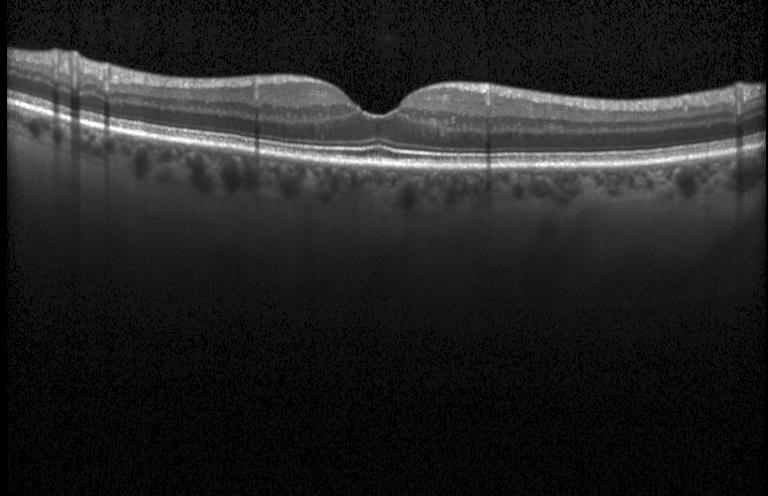

Retinal OCT B-scan · spectral-domain OCT
Finding: no evidence of choroidal neovascularization, diabetic macular edema, or drusen.